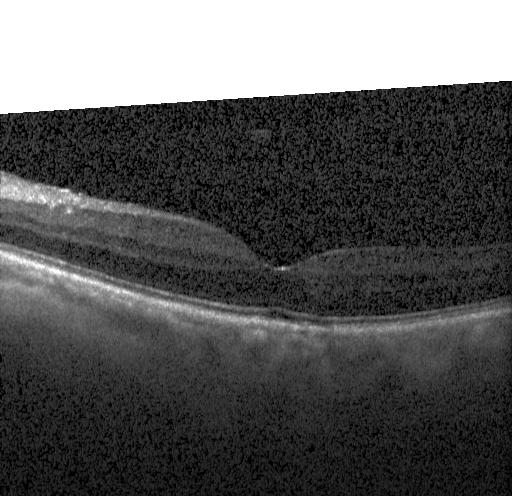 OCT line scan. Horizontal scan through the fovea. Spectral-domain optical coherence tomography. Instrument: Heidelberg Spectralis — The scan shows no choroidal neovascularization, diabetic macular edema, or drusen.